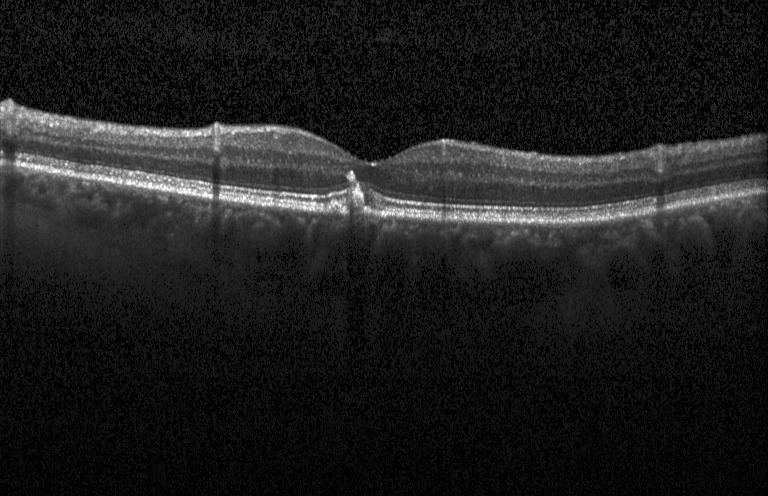
Macular OCT: multiple drusen.